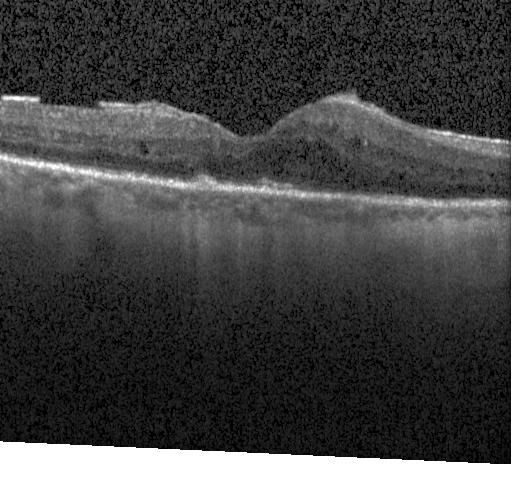 OCT line scan.
Impression: diabetic macular edema (DME).